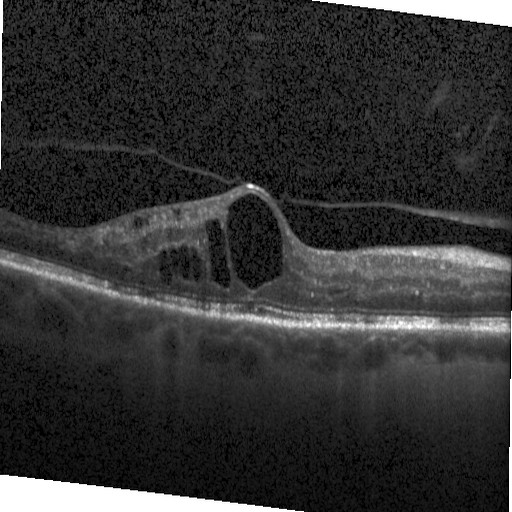

Impression: diabetic macular edema.